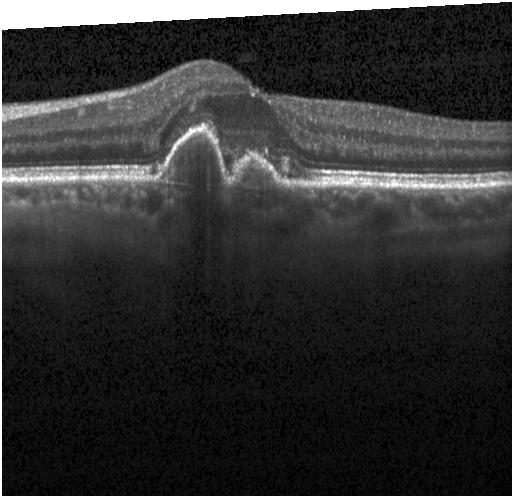 Spectral-domain OCT, instrument: Heidelberg Spectralis, optical coherence tomography B-scan.
Assessment: choroidal neovascularization.